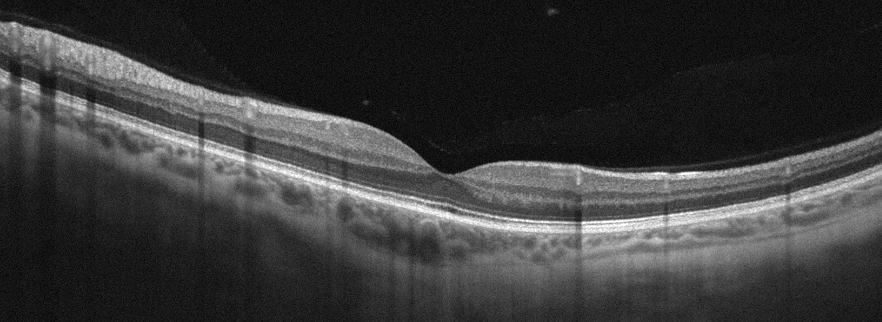 Acquired on an Optovue Avanti RTVue XR. Retinal OCT B-scan. The scan shows absence of AMD, DME, ERM, RAO, RVO, and vitreomacular interface disease.